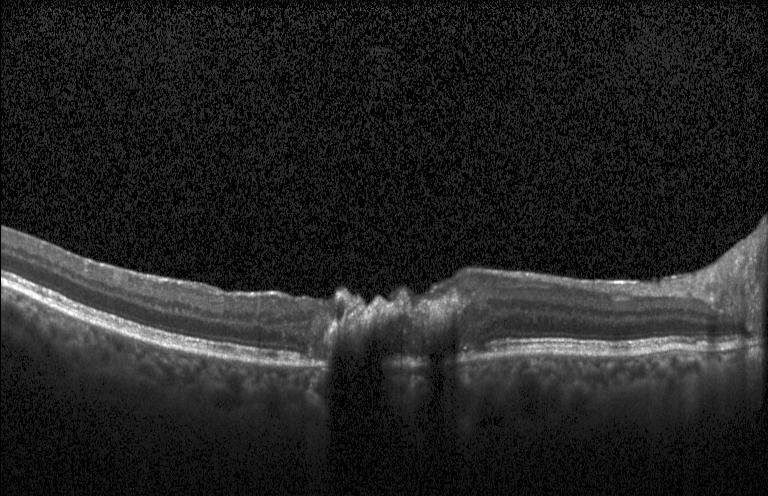 Horizontal scan through the fovea, optical coherence tomography B-scan, Heidelberg Spectralis OCT system — This B-scan demonstrates a choroidal neovascular membrane.